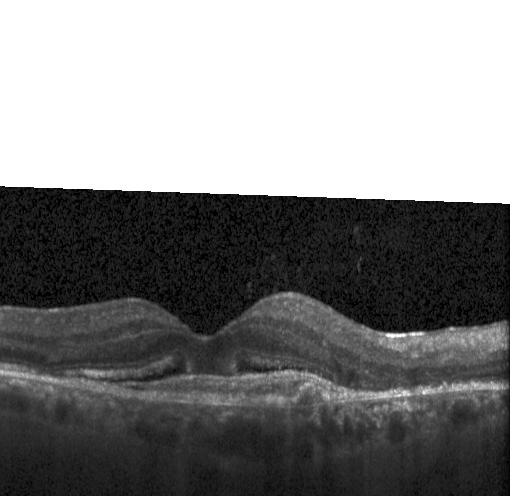
Impression: CNV.